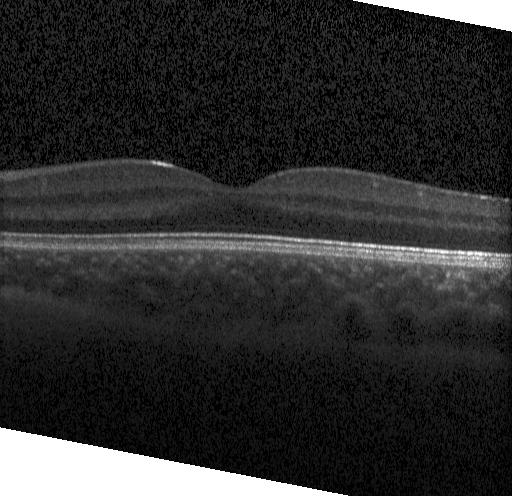
Optical coherence tomography scan, spectral-domain optical coherence tomography, centered on the fovea. Impression: no CNV, no DME, and no drusen.